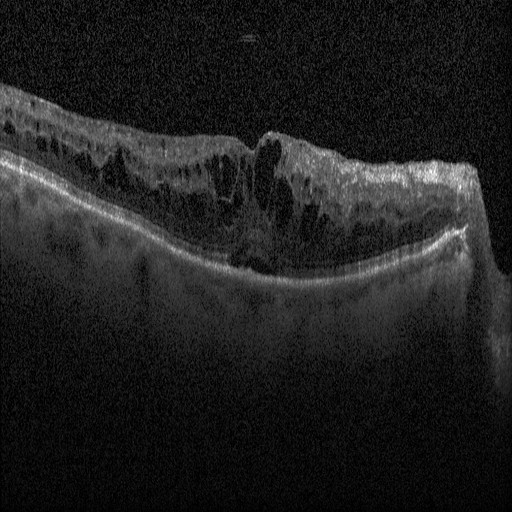
DME.